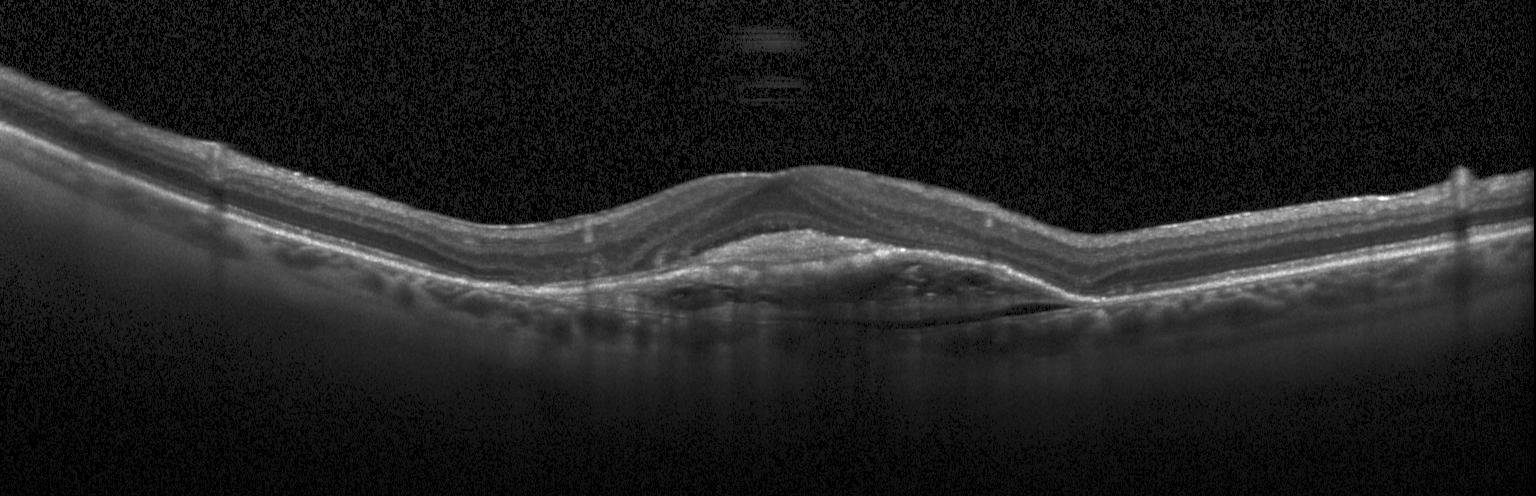 OCT finding: choroidal neovascularization (CNV).